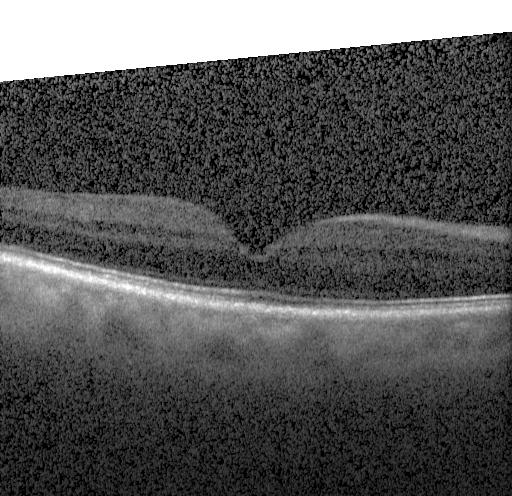

SD-OCT · optical coherence tomography scan. Dx: no CNV, no DME, and no drusen.